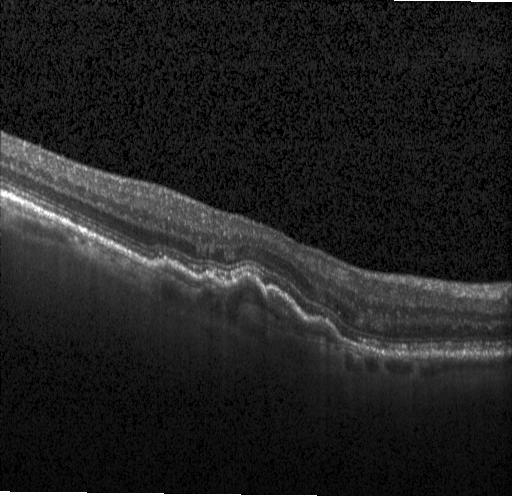
Diagnosis: choroidal neovascularization (CNV).